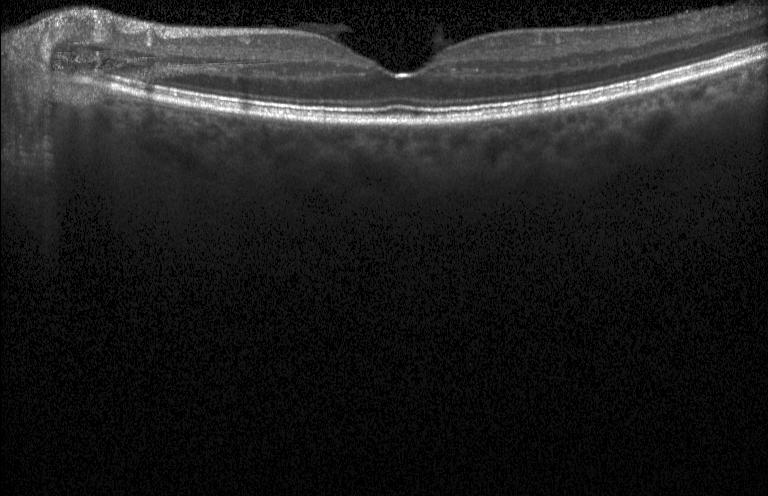
Fovea-centered, SD-OCT, optical coherence tomography B-scan.
Assessment: no choroidal neovascularization, diabetic macular edema, or drusen.